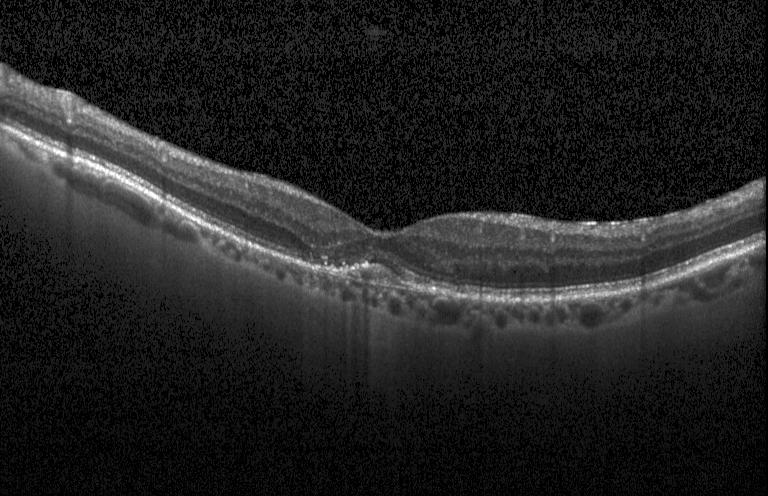

Through the macula, retinal OCT cross-section, instrument: Heidelberg Spectralis
Assessment: a choroidal neovascular membrane.